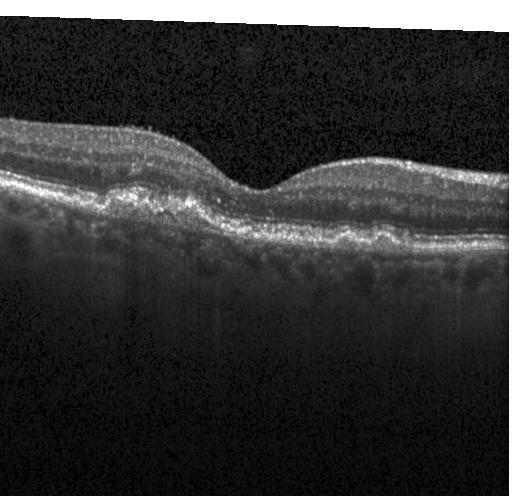
OCT B-scan. This B-scan demonstrates choroidal neovascularization.